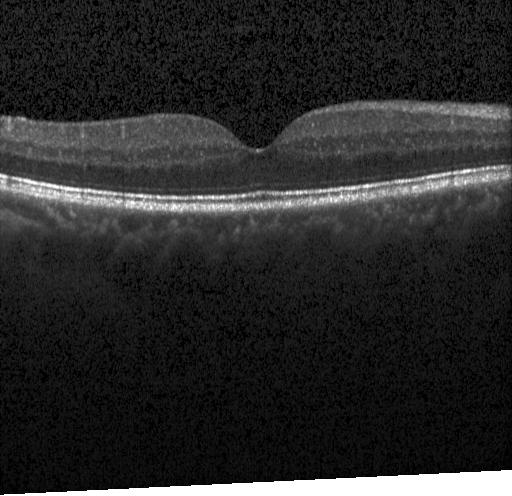
Spectral-domain OCT B-scan: no evidence of choroidal neovascularization, diabetic macular edema, or drusen.